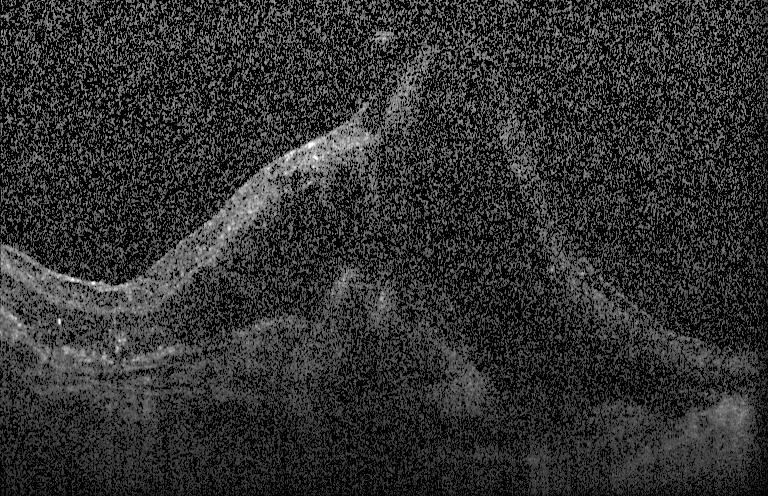

The scan shows CNV.